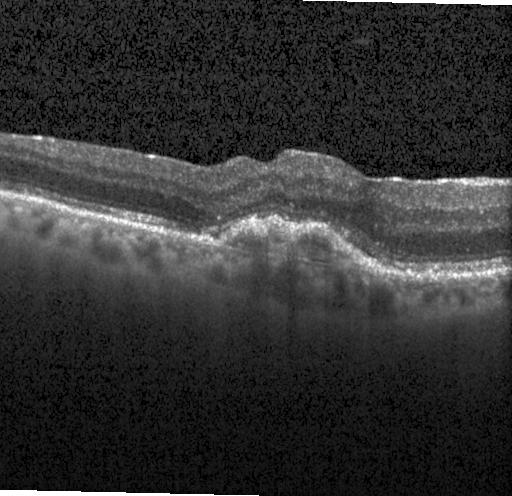 Diagnosis: a choroidal neovascular membrane.